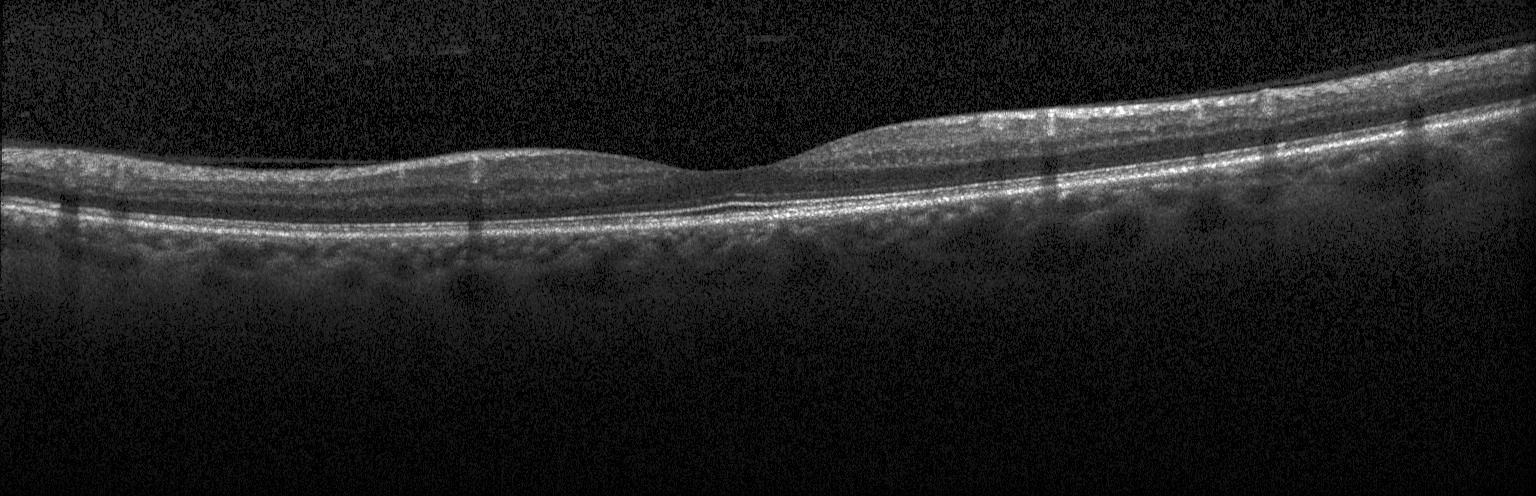
Heidelberg Spectralis OCT system; through the macula; retinal OCT cross-section; spectral-domain optical coherence tomography — Diagnosis: no CNV, no DME, and no drusen.